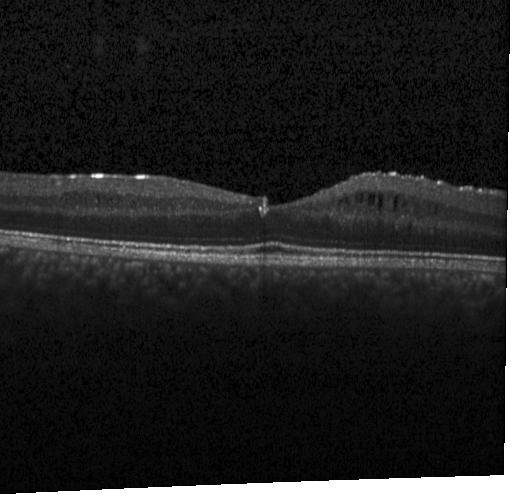 Macular OCT: DME.